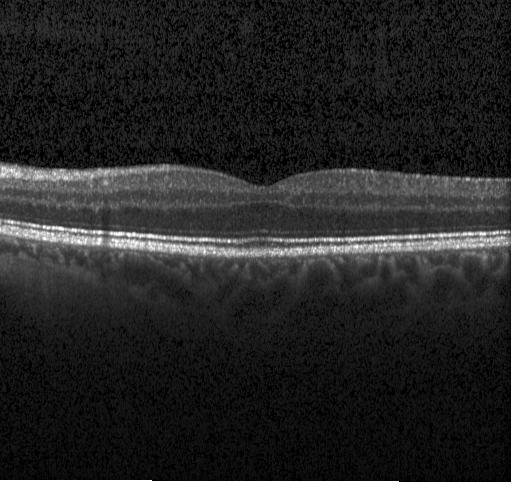 Heidelberg Spectralis. OCT B-scan. Spectral-domain OCT.
No choroidal neovascularization, diabetic macular edema, or drusen.